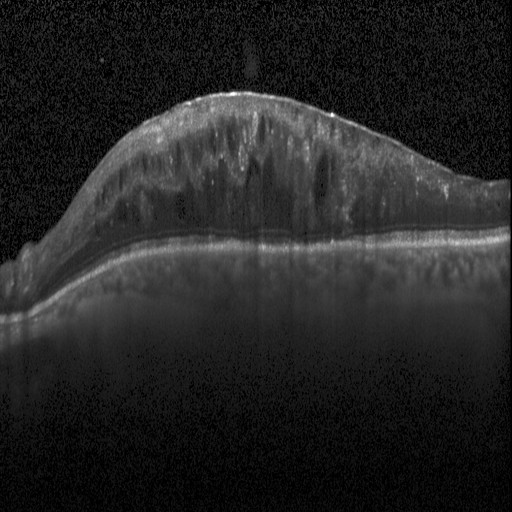

Dx: diabetic macular edema.